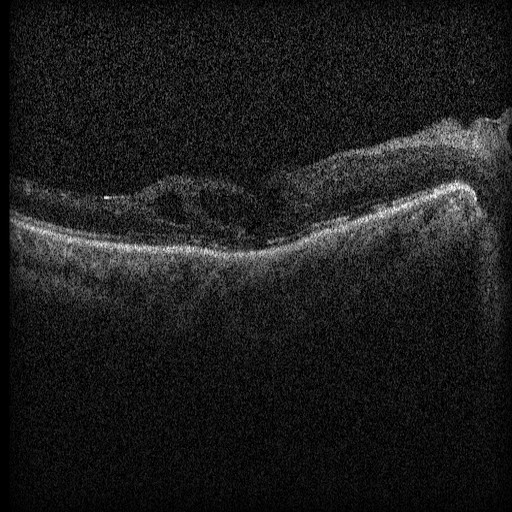 Instrument: Heidelberg Spectralis. Spectral-domain OCT. Fovea-centered. Optical coherence tomography scan — Dx: DME.